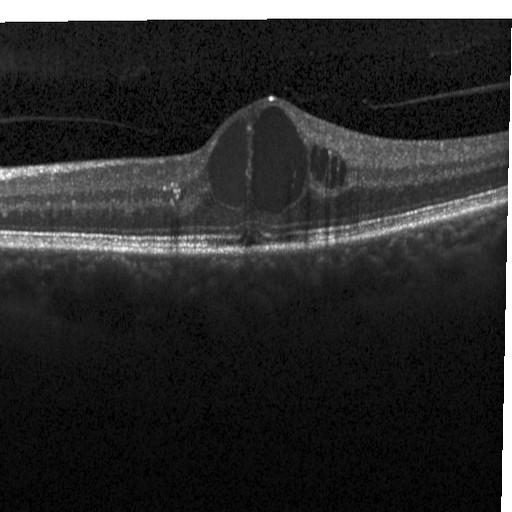
The scan shows diabetic macular edema.